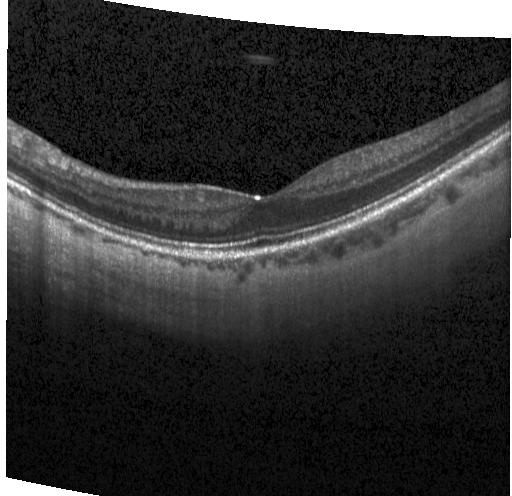 Macular OCT: no CNV, DME, or drusen.